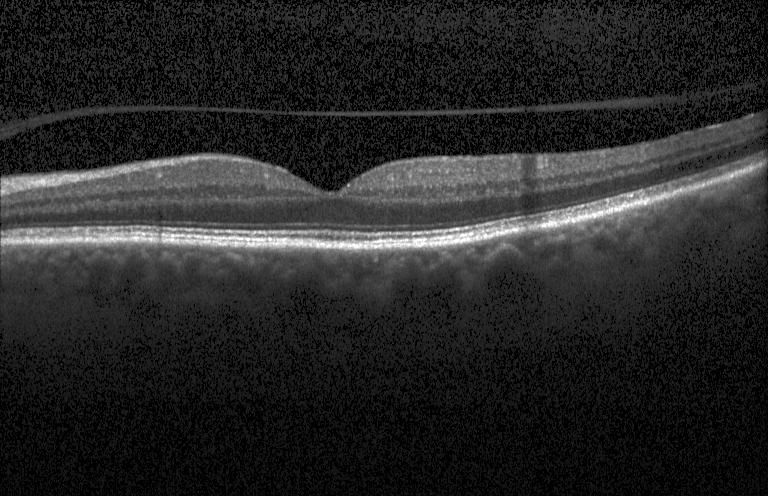

Spectral-domain OCT · centered on the fovea · OCT B-scan · Heidelberg Spectralis OCT system.
Assessment: no evidence of CNV, DME, or drusen.